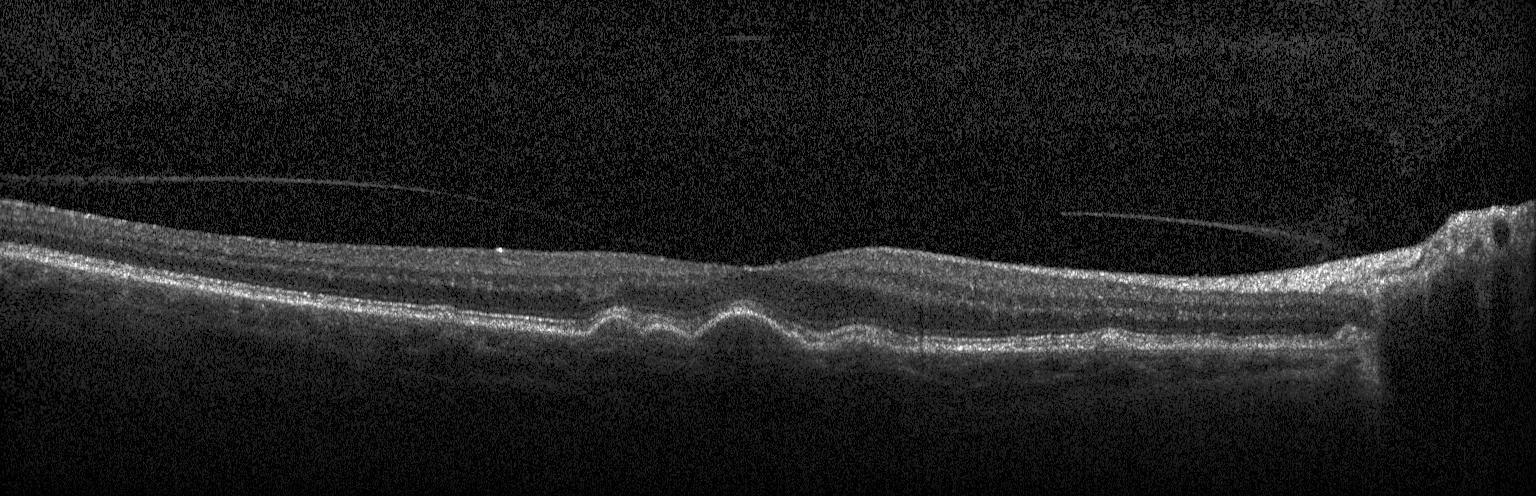

This B-scan demonstrates a choroidal neovascular membrane.